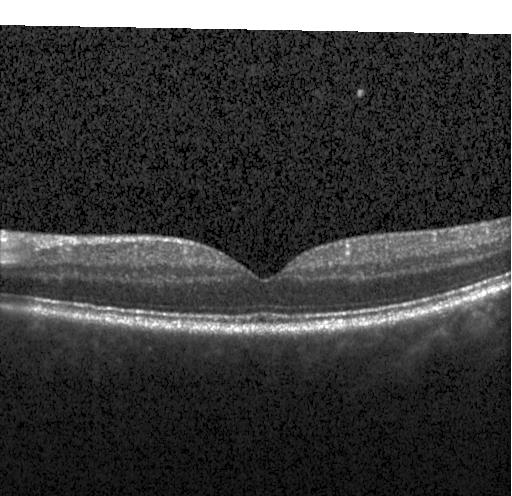

OCT B-scan showing neither choroidal neovascularization, diabetic macular edema, nor drusen.